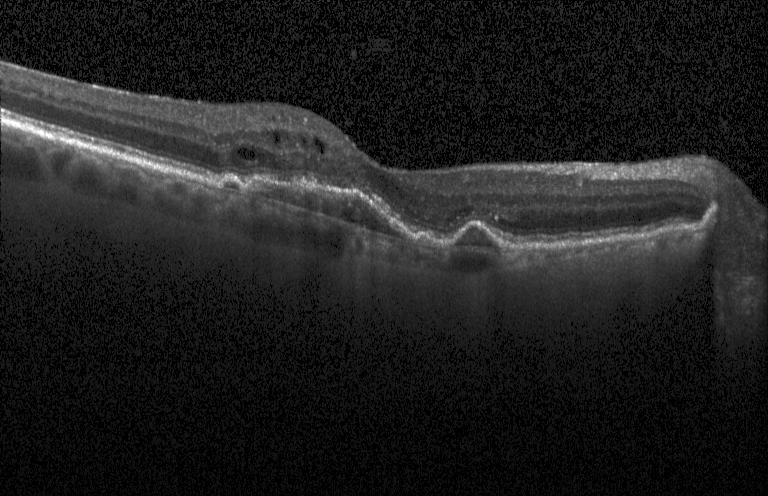 Diagnosis: choroidal neovascularization.